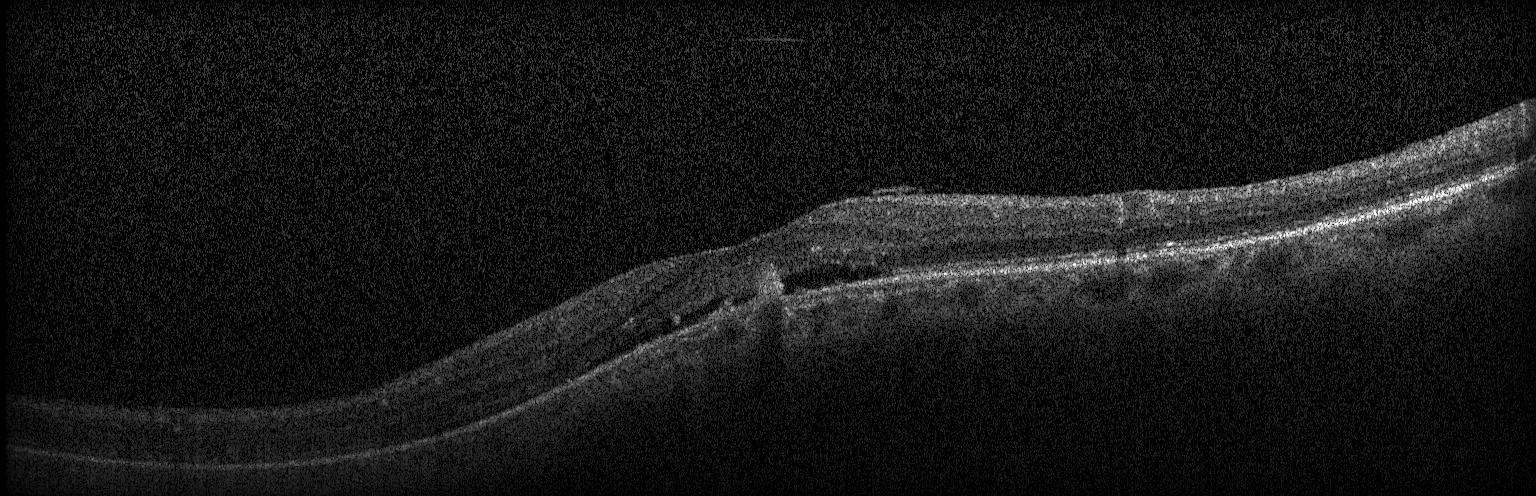

Finding: CNV.